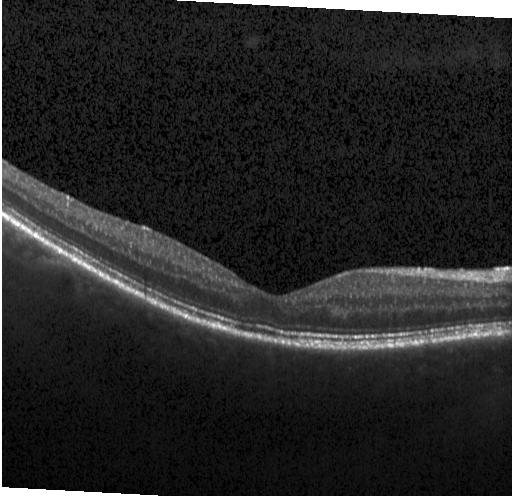 Retinal OCT cross-section. Acquired on a Heidelberg Spectralis.
Impression: no choroidal neovascularization, diabetic macular edema, or drusen.